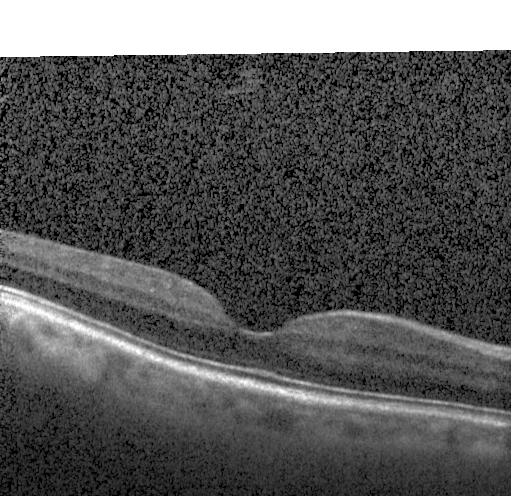
Horizontal scan through the fovea. Heidelberg Spectralis OCT system. OCT line scan.
Neither CNV, DME, nor drusen.